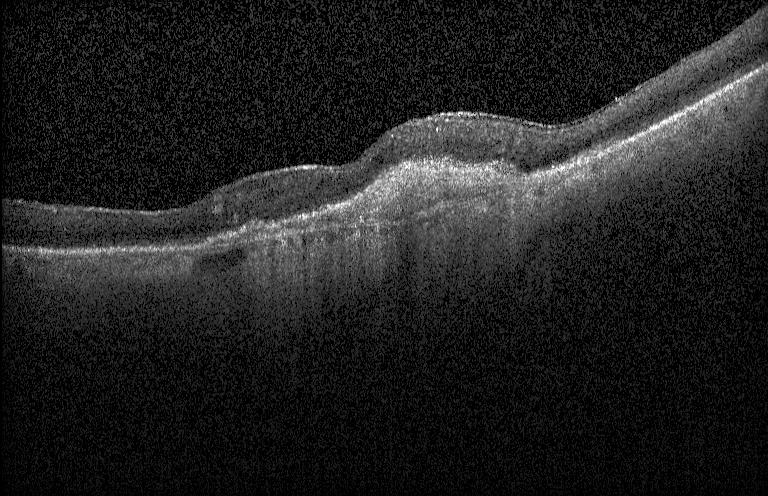
This B-scan demonstrates choroidal neovascularization.